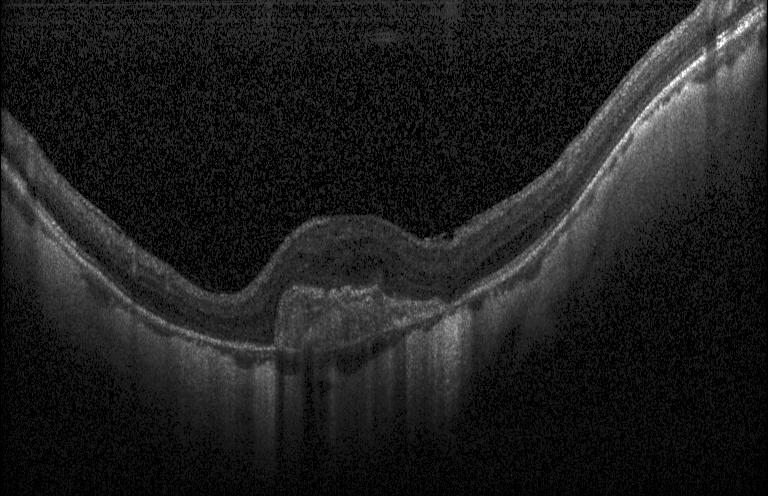

Through the macula · retinal OCT B-scan. The scan shows choroidal neovascularization.